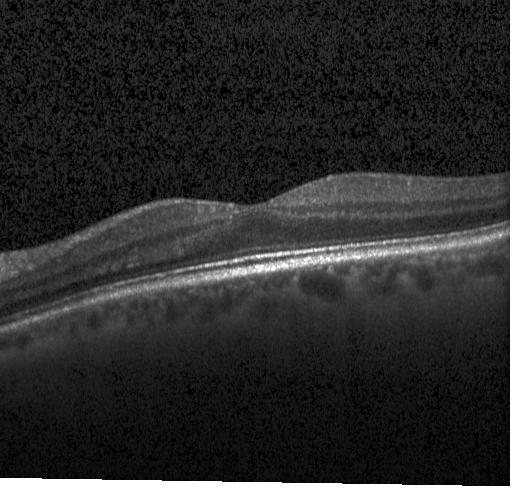 Retinal OCT B-scan. Impression: neither choroidal neovascularization, diabetic macular edema, nor drusen.